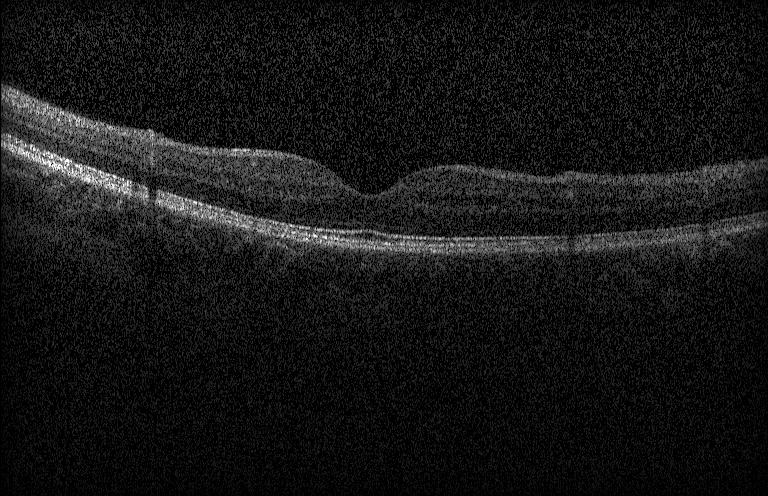

OCT line scan. OCT finding: no evidence of choroidal neovascularization, diabetic macular edema, or drusen.